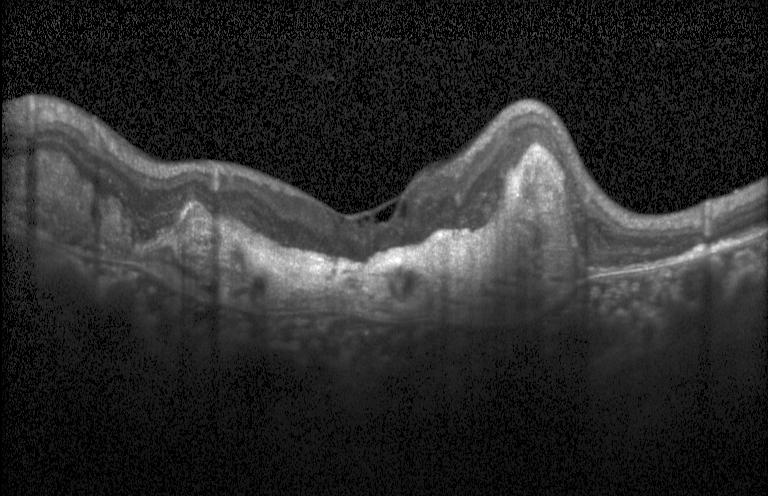
SD-OCT, retinal OCT cross-section, centered on the fovea. Impression: a choroidal neovascular membrane.